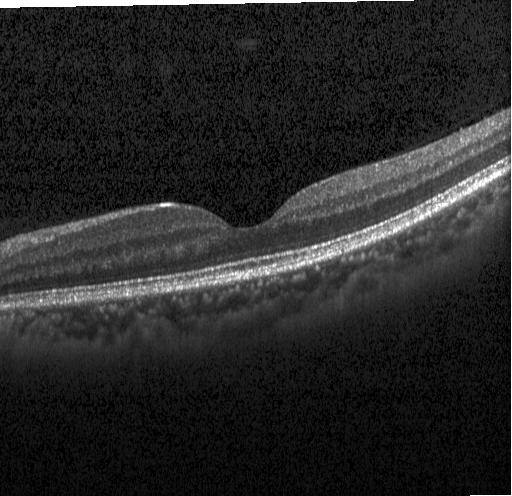
OCT line scan; instrument: Heidelberg Spectralis — Finding: no CNV, no DME, and no drusen.